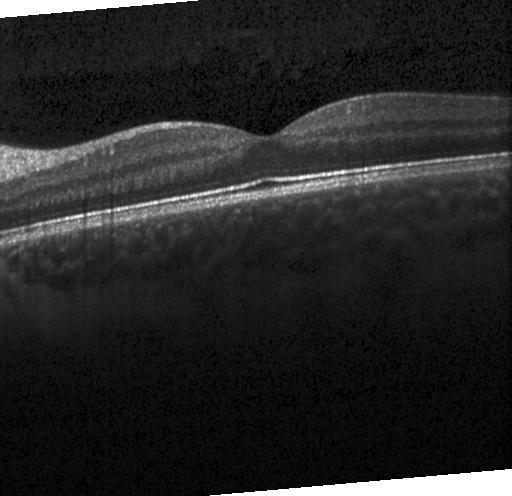 Optical coherence tomography B-scan, Heidelberg Spectralis, spectral-domain optical coherence tomography — The scan shows neither choroidal neovascularization, diabetic macular edema, nor drusen.